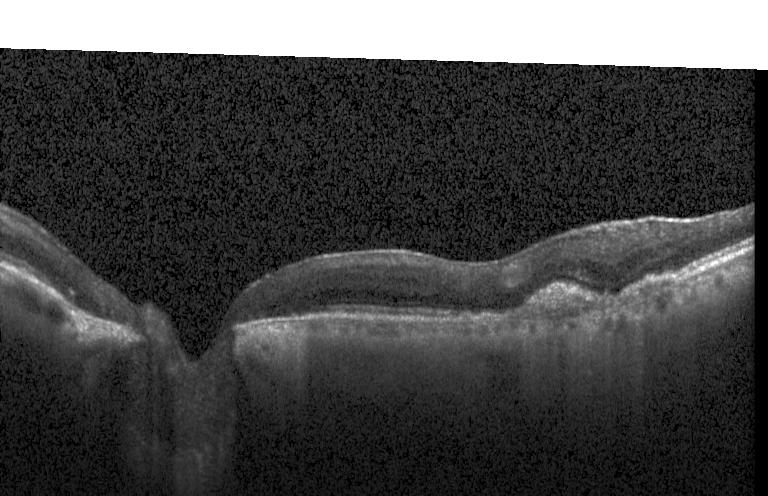

Impression: a choroidal neovascular membrane.